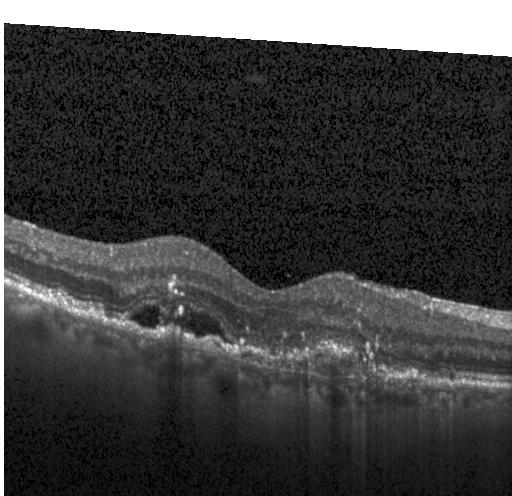

Retinal OCT B-scan; through the macula; spectral-domain optical coherence tomography
A choroidal neovascular membrane.